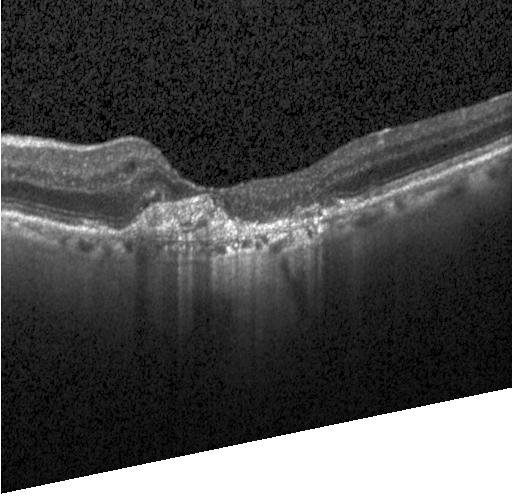
Impression: CNV.